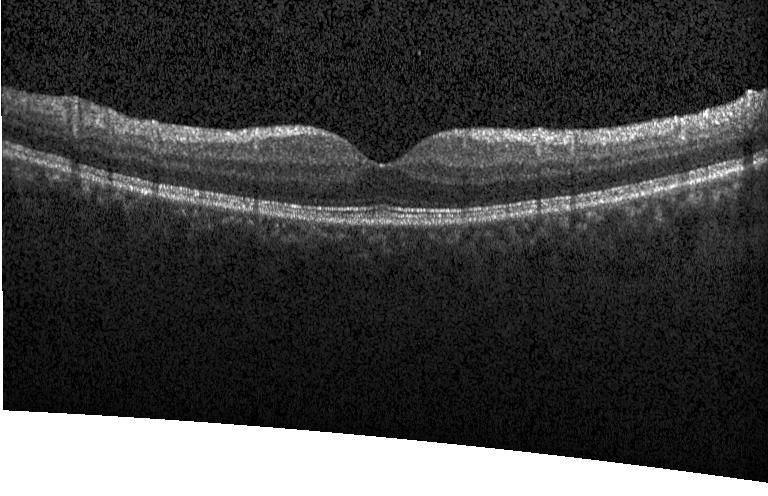

Through the macula · OCT line scan. Finding: no CNV, DME, or drusen.